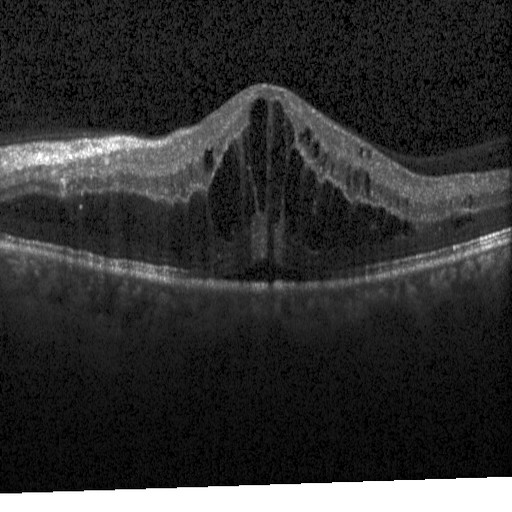
Spectral-domain OCT; retinal OCT cross-section; acquired on a Heidelberg Spectralis; fovea-centered
Macular OCT: diabetic macular edema (DME).